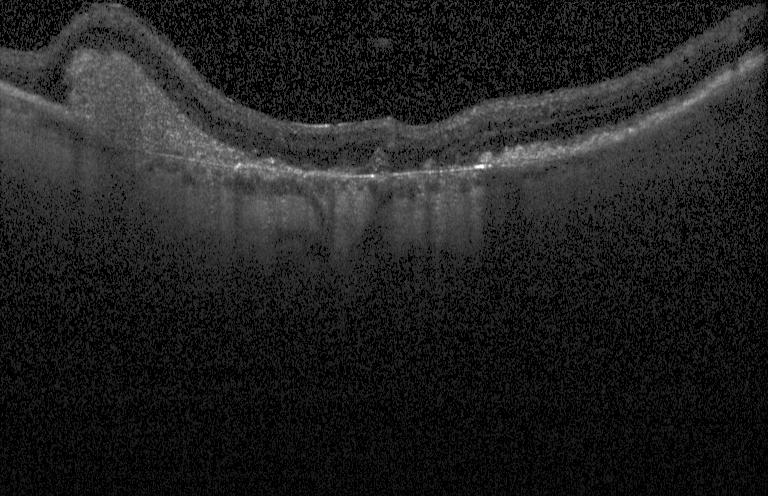 OCT B-scan · fovea-centered · spectral-domain OCT
Diagnosis: CNV.